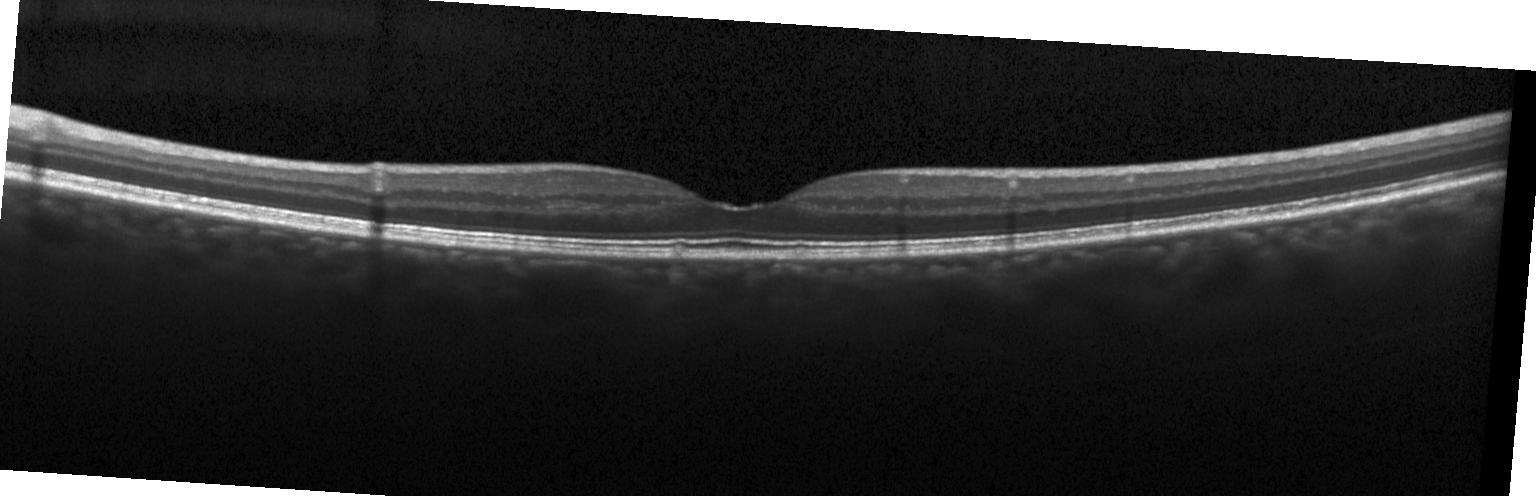 Spectral-domain optical coherence tomography; optical coherence tomography B-scan
Diagnosis: no choroidal neovascularization, no diabetic macular edema, and no drusen.